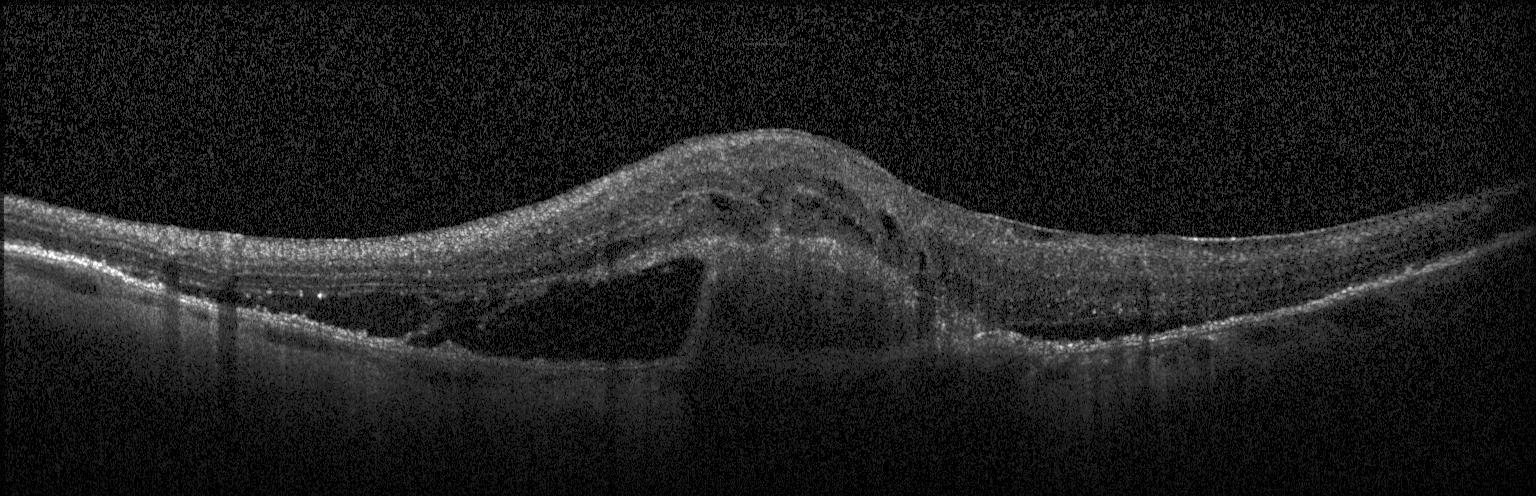 Impression: a choroidal neovascular membrane.